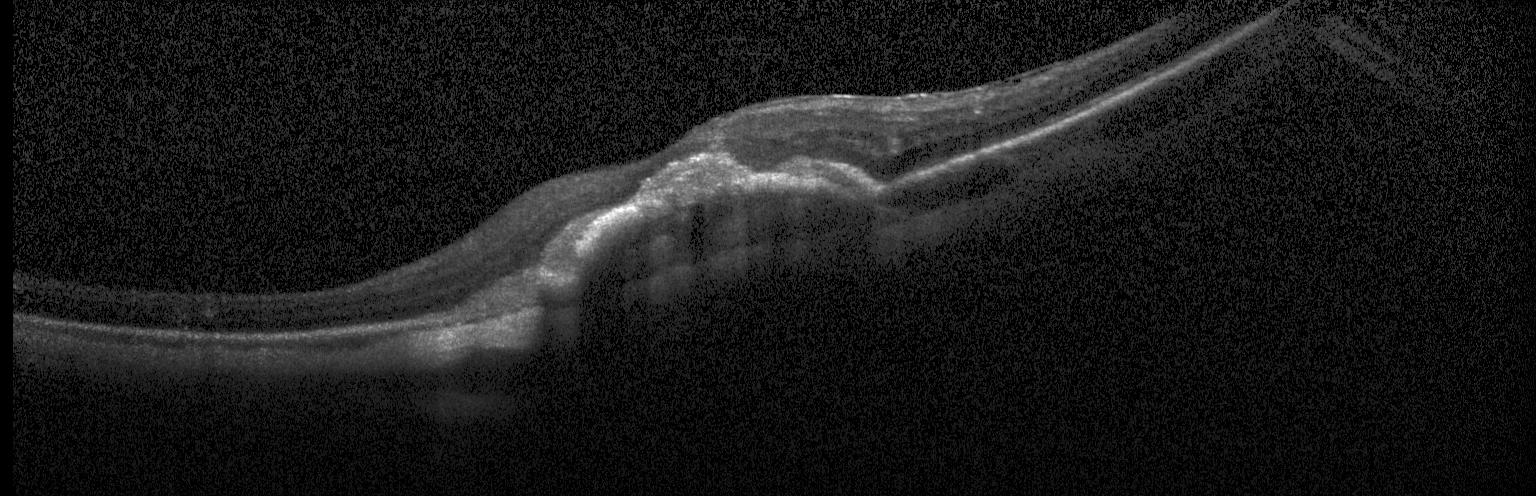
Retinal OCT cross-section. Acquired on a Heidelberg Spectralis. SD-OCT. Horizontal scan through the fovea. Impression: a choroidal neovascular membrane.